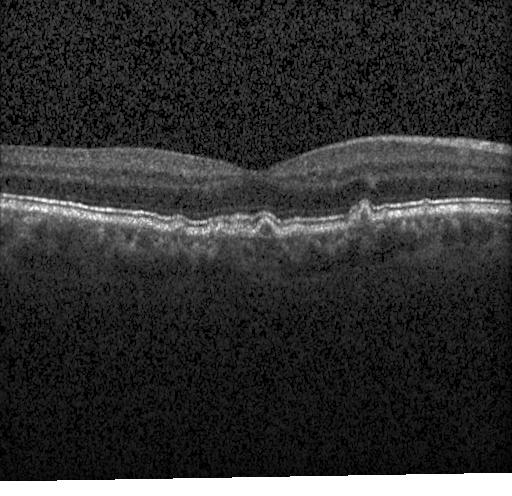 Macular scan, instrument: Heidelberg Spectralis, retinal OCT B-scan, SD-OCT. Finding: multiple drusen.